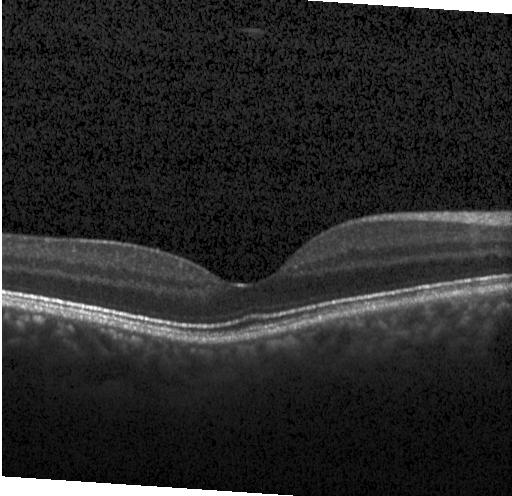

Optical coherence tomography scan, spectral-domain optical coherence tomography, fovea-centered — The scan shows no CNV, no DME, and no drusen.